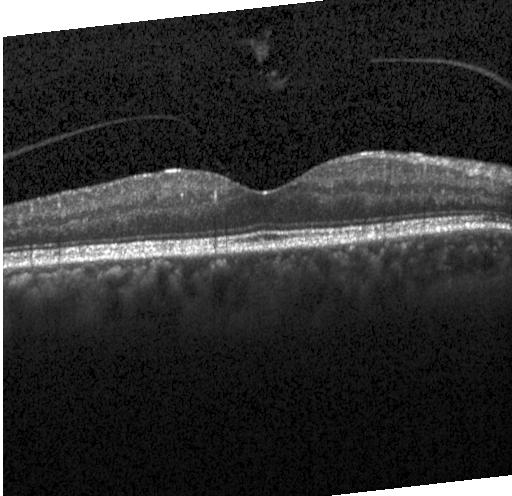

Macular scan; acquired on a Heidelberg Spectralis; spectral-domain OCT; optical coherence tomography B-scan — Assessment: no evidence of choroidal neovascularization, diabetic macular edema, or drusen.